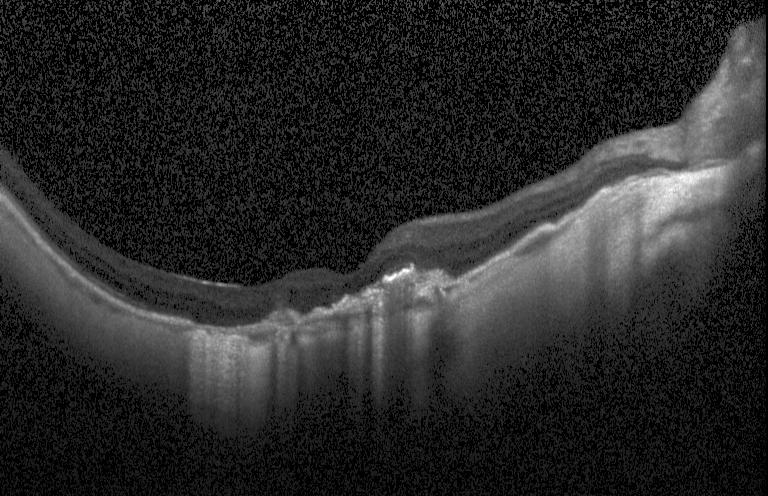
OCT B-scan.
A choroidal neovascular membrane.